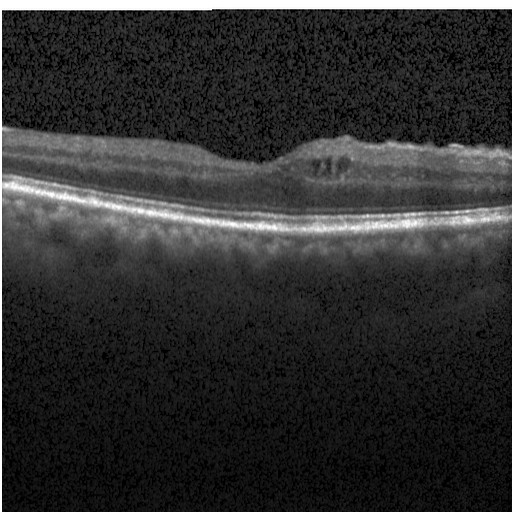

Acquired on a Heidelberg Spectralis, optical coherence tomography B-scan.
Impression: DME.